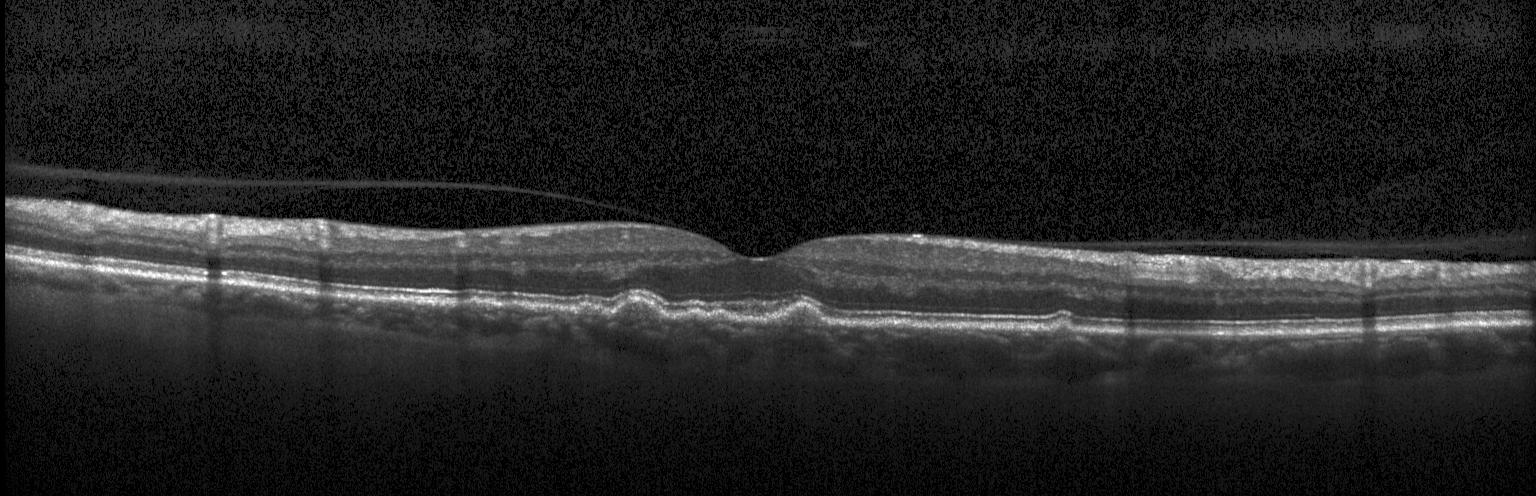

OCT B-scan showing multiple drusen.